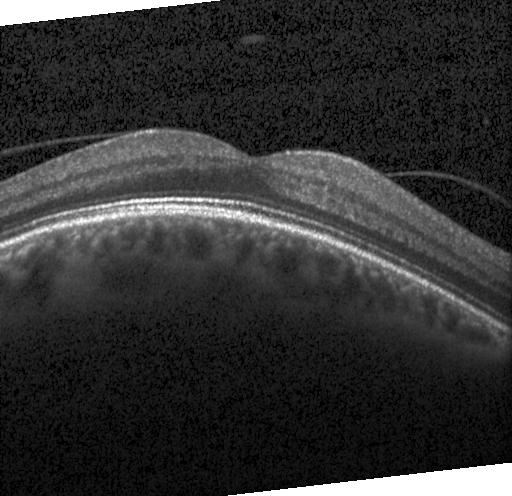

Acquired on a Heidelberg Spectralis; fovea-centered; retinal OCT B-scan — Finding: no CNV, DME, or drusen.